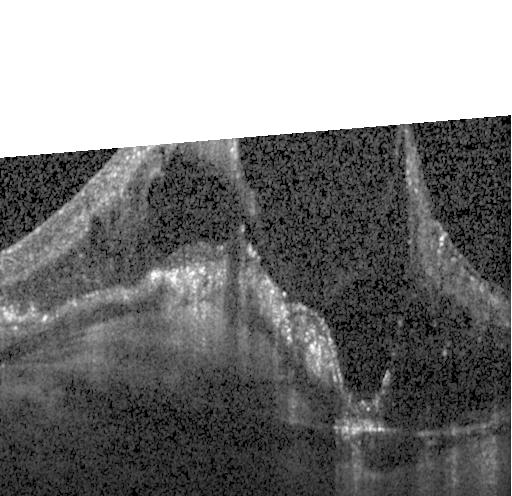
Retinal OCT cross-section.
Macular OCT: CNV.